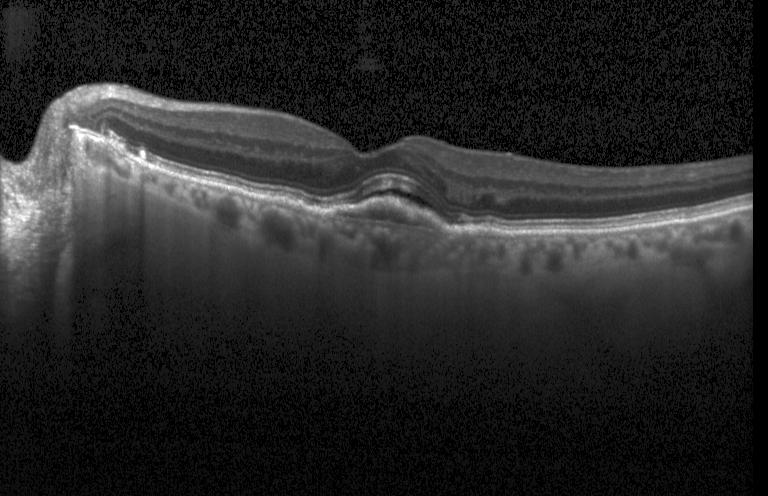 Heidelberg Spectralis; optical coherence tomography scan; horizontal scan through the fovea — Finding: a choroidal neovascular membrane.